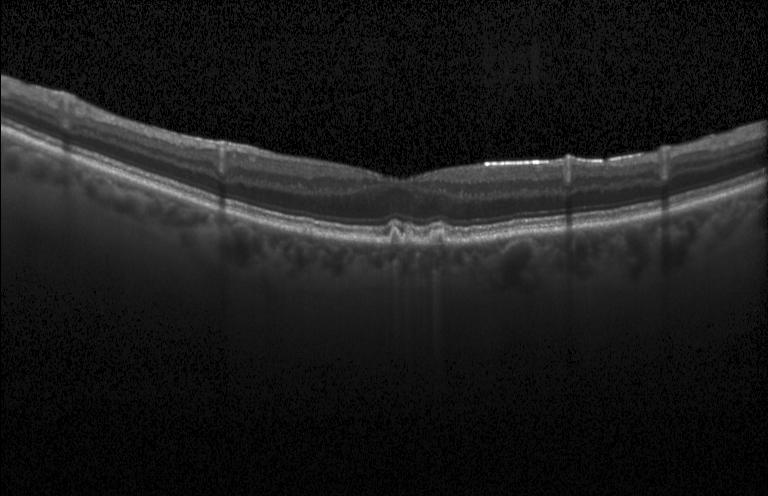

Impression: sub-RPE drusenoid deposits.